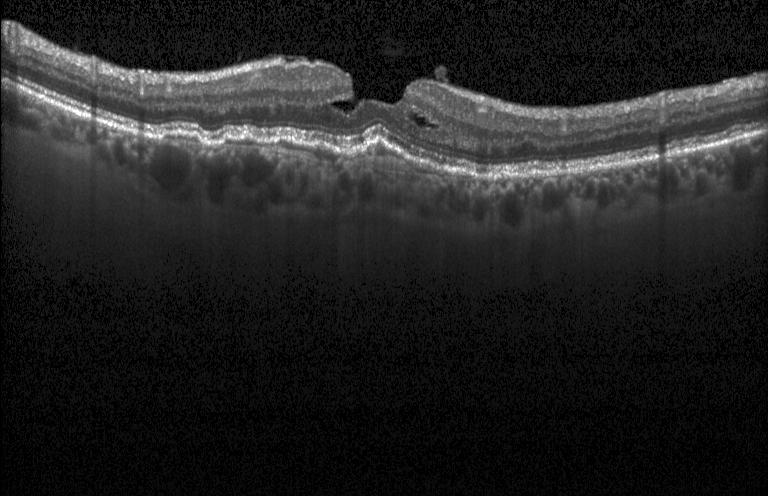 OCT B-scan. Spectral-domain OCT. Instrument: Heidelberg Spectralis. Centered on the fovea — Macular OCT: a choroidal neovascular membrane.